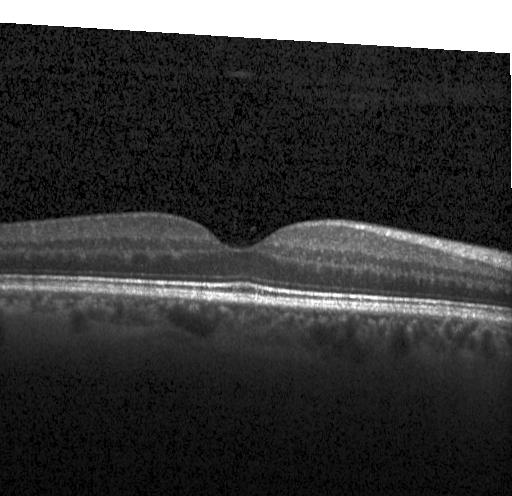 Diagnosis: no CNV, no DME, and no drusen.